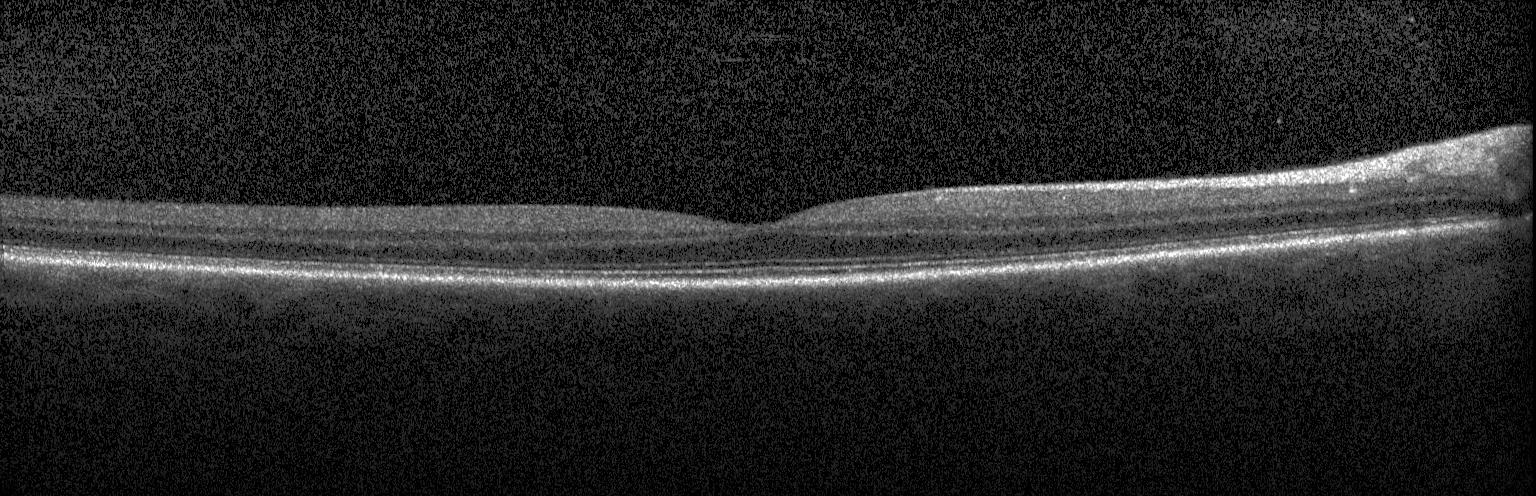 Spectral-domain OCT, OCT B-scan, through the macula, acquired on a Heidelberg Spectralis.
Finding: no choroidal neovascularization, diabetic macular edema, or drusen.